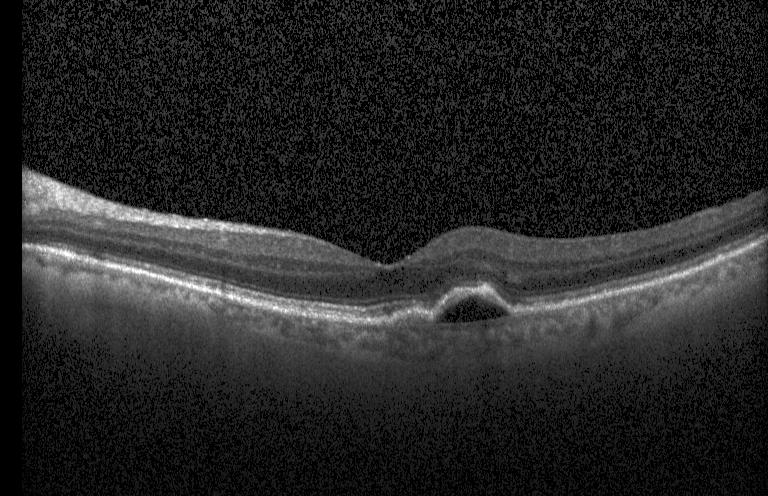

OCT line scan; acquired on a Heidelberg Spectralis.
Macular OCT: a choroidal neovascular membrane.